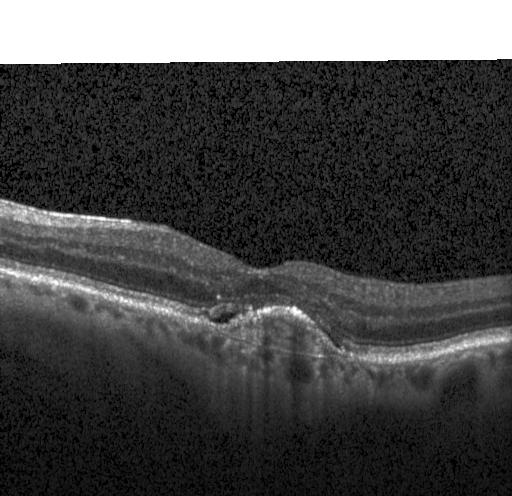
Acquired on a Heidelberg Spectralis, spectral-domain optical coherence tomography, OCT line scan, fovea-centered. Diagnosis: a choroidal neovascular membrane.